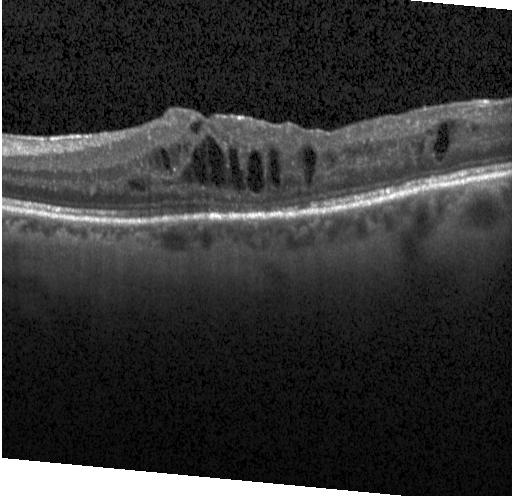 Assessment: diabetic macular edema (DME).